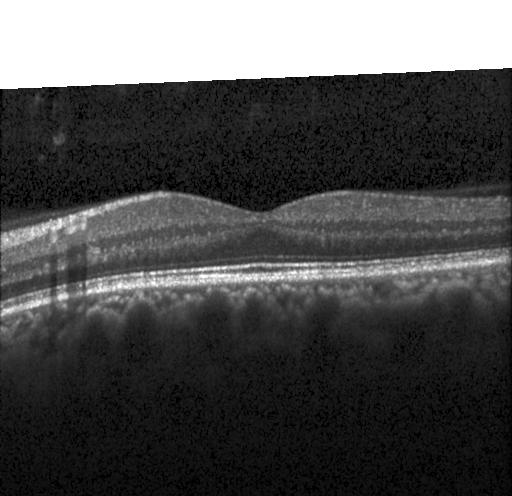

Heidelberg Spectralis OCT system; OCT line scan; fovea-centered — Assessment: no choroidal neovascularization, diabetic macular edema, or drusen.